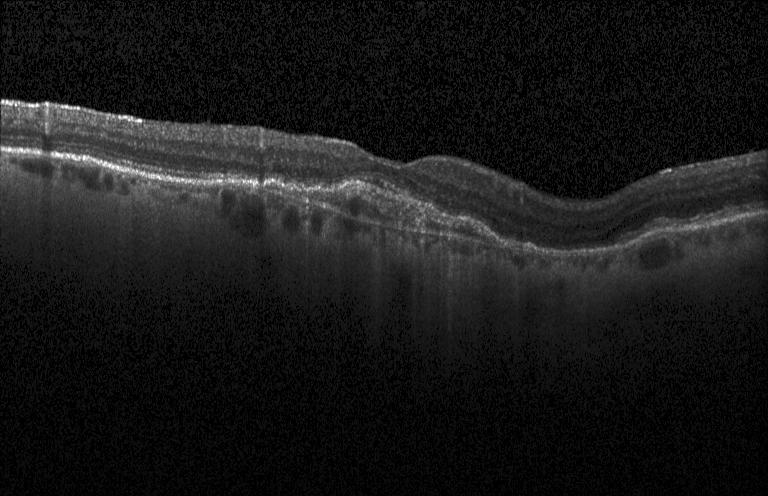 Finding: choroidal neovascularization.